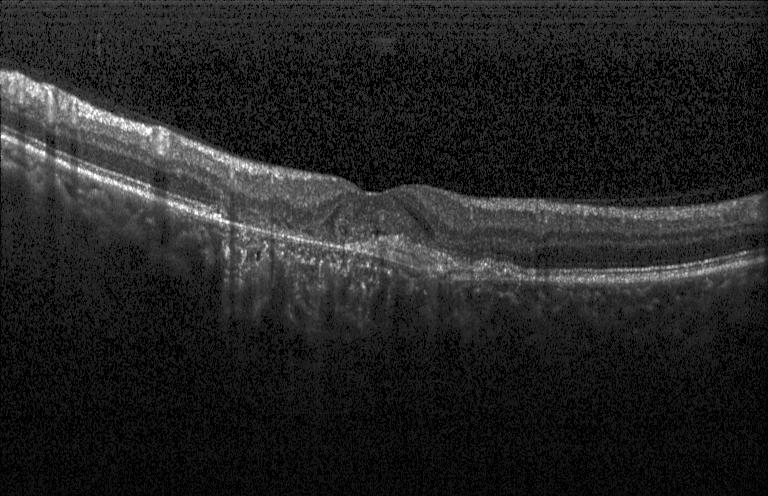

OCT B-scan · instrument: Heidelberg Spectralis.
Finding: a choroidal neovascular membrane.